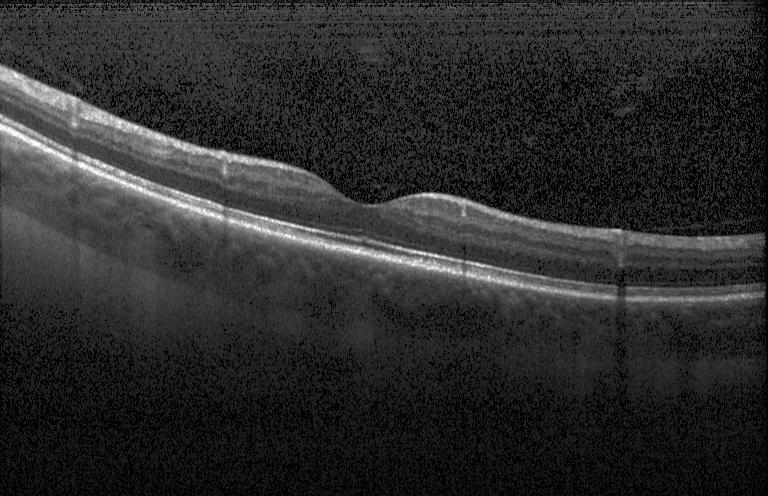

SD-OCT · retinal OCT B-scan. Diagnosis: no evidence of choroidal neovascularization, diabetic macular edema, or drusen.